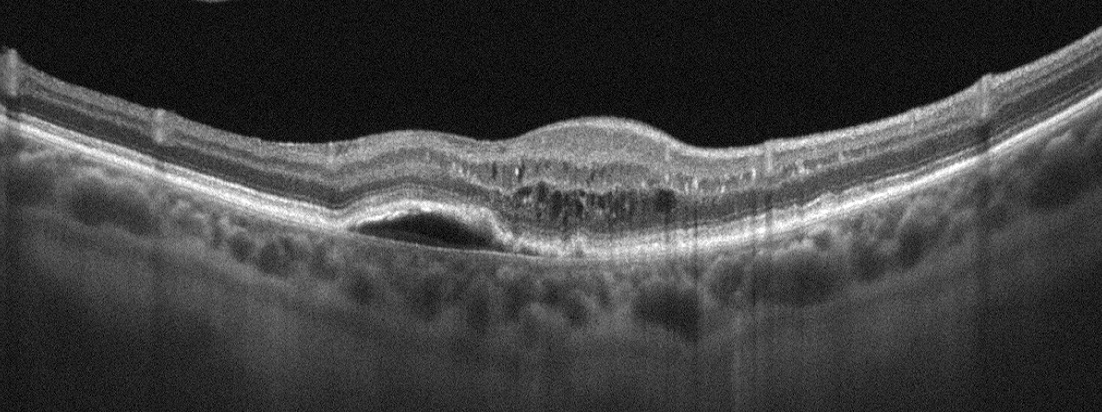
Optical coherence tomography scan
This B-scan demonstrates age-related macular degeneration (AMD).